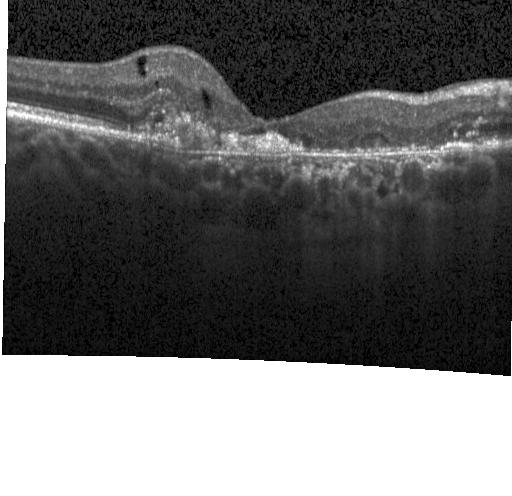

Macular OCT: a choroidal neovascular membrane.